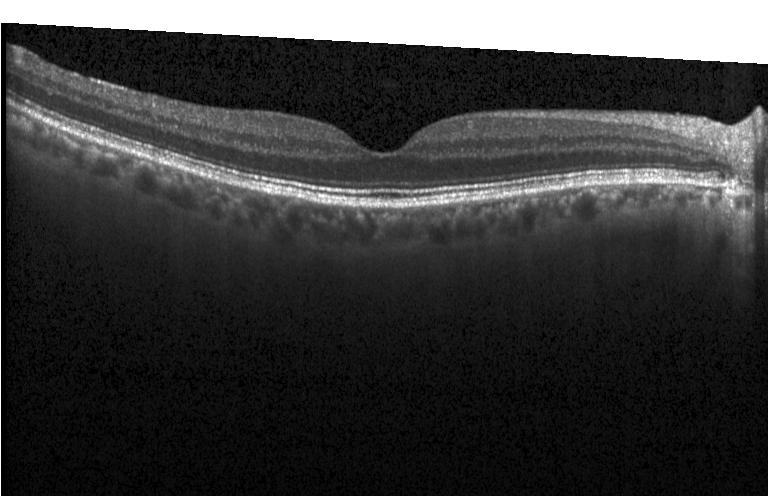 Optical coherence tomography scan
The scan shows no evidence of choroidal neovascularization, diabetic macular edema, or drusen.